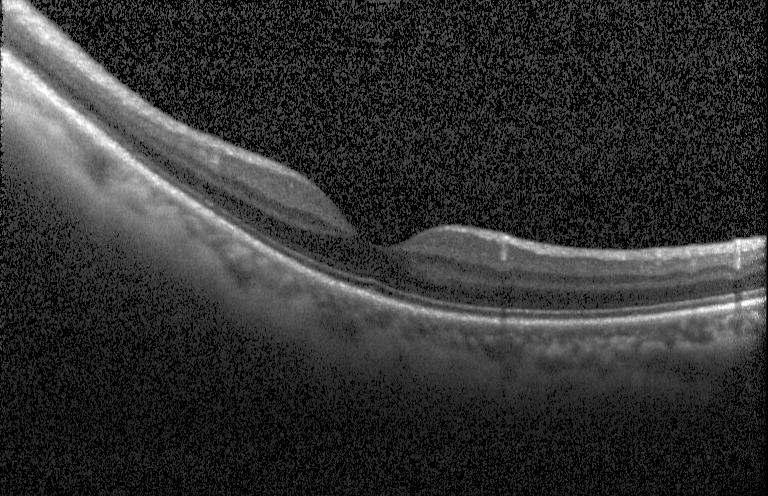
OCT finding: no choroidal neovascularization, no diabetic macular edema, and no drusen.